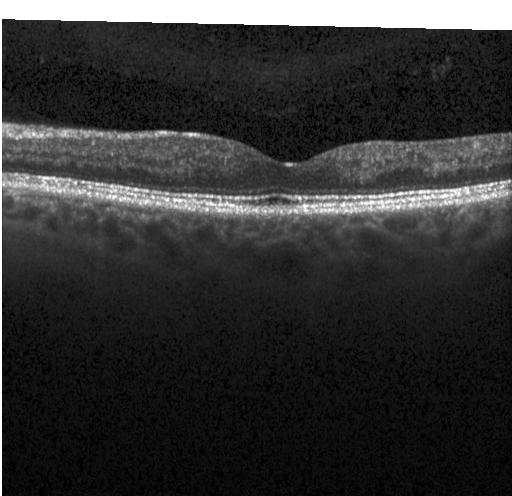
Spectral-domain optical coherence tomography, OCT B-scan.
Macular OCT: neither choroidal neovascularization, diabetic macular edema, nor drusen.